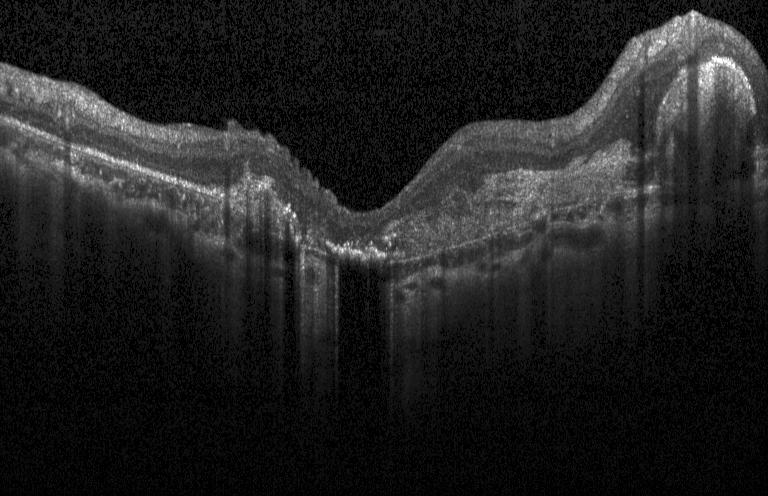 OCT B-scan. CNV.